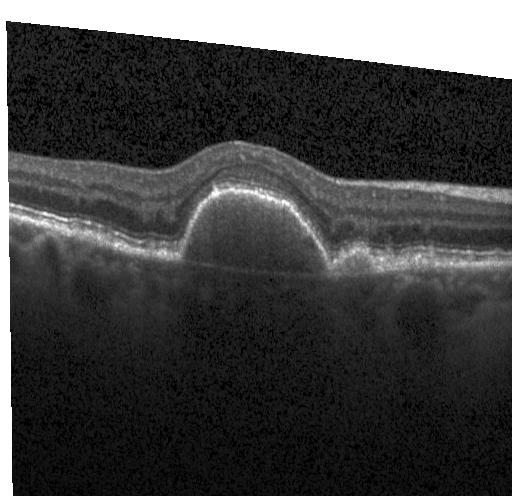

OCT B-scan. Dx: CNV.